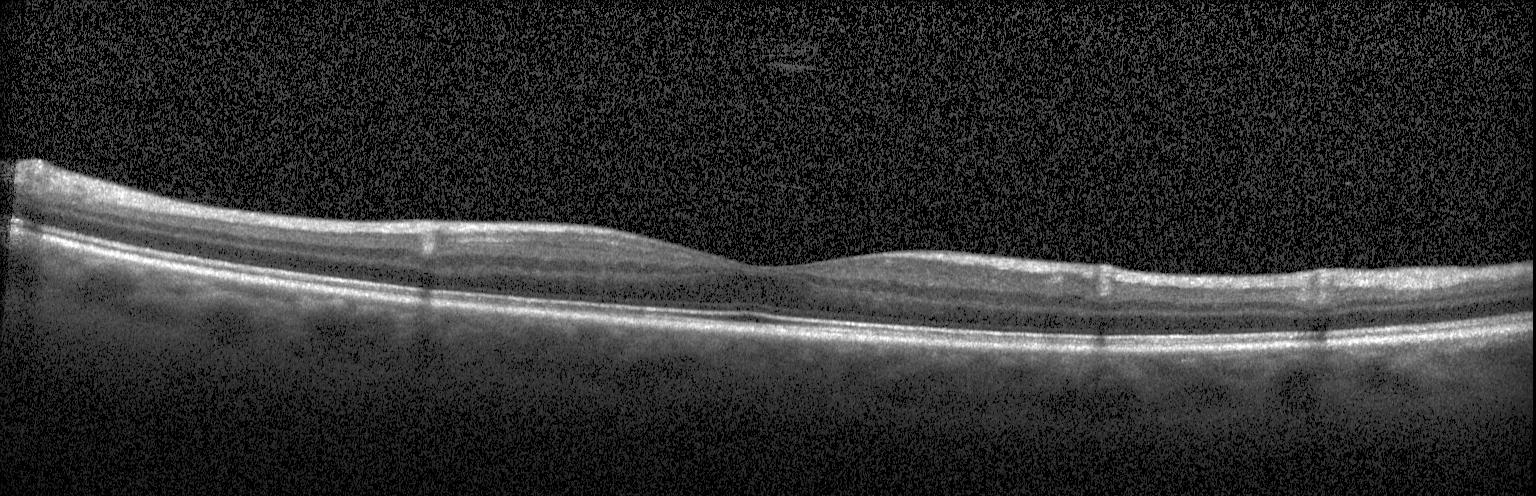 Finding: no evidence of choroidal neovascularization, diabetic macular edema, or drusen.